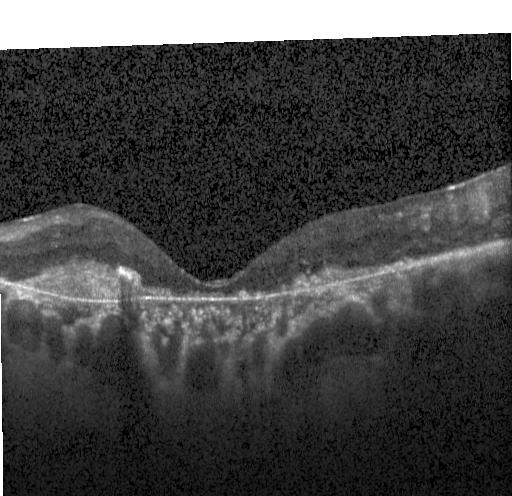

Impression: choroidal neovascularization.